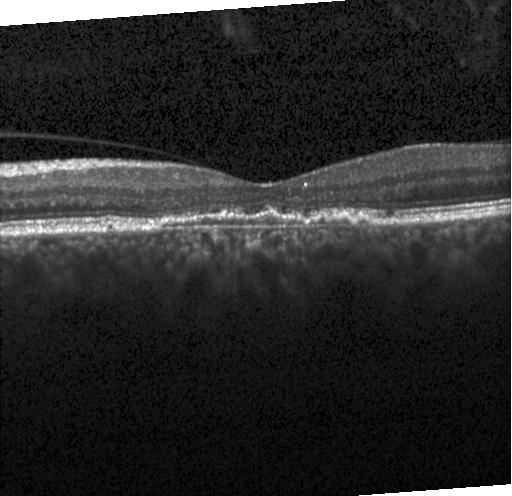 Choroidal neovascularization (CNV).